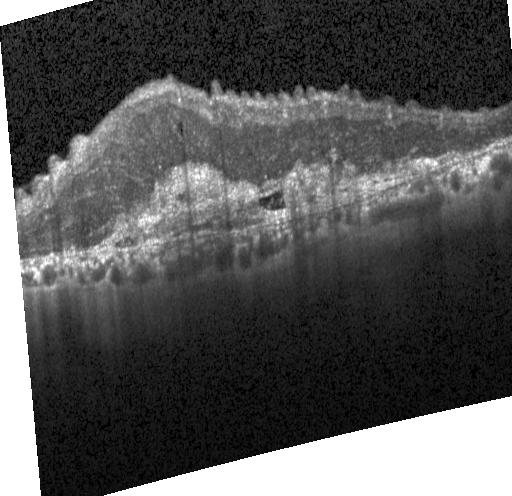

Diagnosis: a choroidal neovascular membrane.